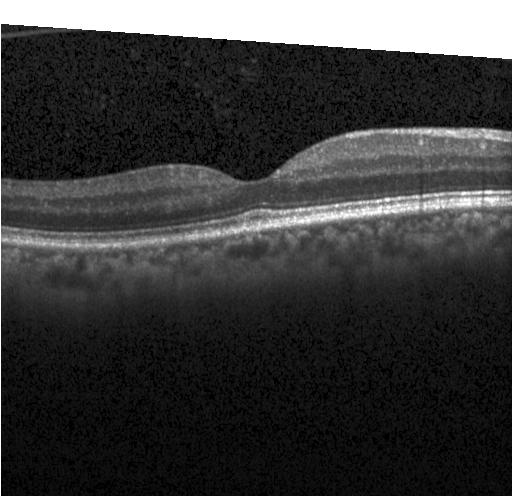 Through the macula, Heidelberg Spectralis, retinal OCT cross-section, spectral-domain optical coherence tomography — Finding: no choroidal neovascularization, no diabetic macular edema, and no drusen.